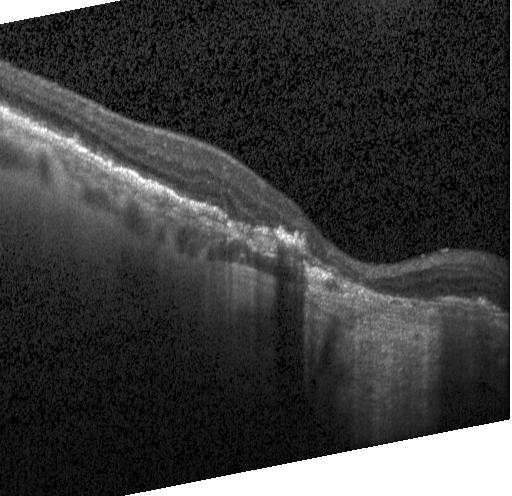
Spectral-domain OCT B-scan: a choroidal neovascular membrane.